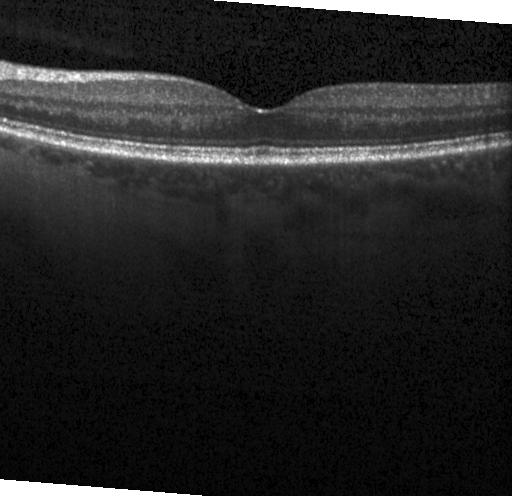
Optical coherence tomography B-scan. Through the macula. Spectral-domain optical coherence tomography. Instrument: Heidelberg Spectralis. Finding: no choroidal neovascularization, diabetic macular edema, or drusen.